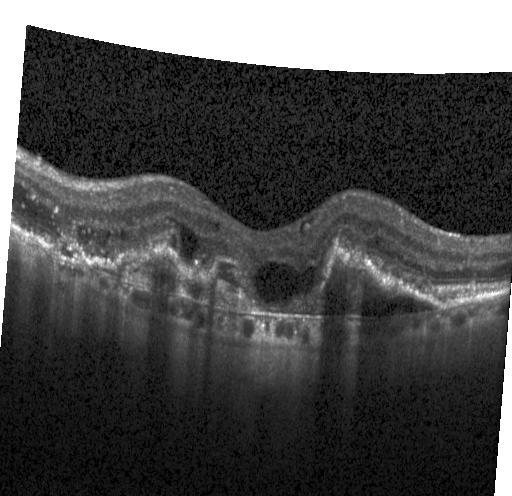
Spectral-domain optical coherence tomography · acquired on a Heidelberg Spectralis · centered on the fovea · retinal OCT cross-section
This B-scan demonstrates a choroidal neovascular membrane.